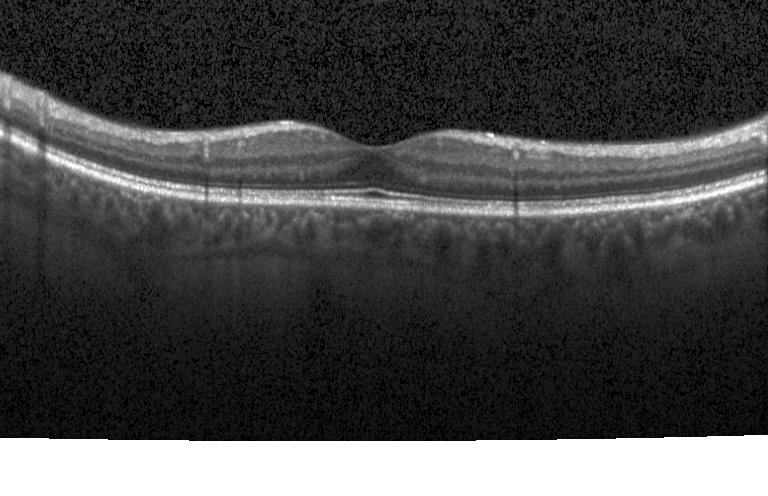 OCT B-scan — Diagnosis: no evidence of CNV, DME, or drusen.